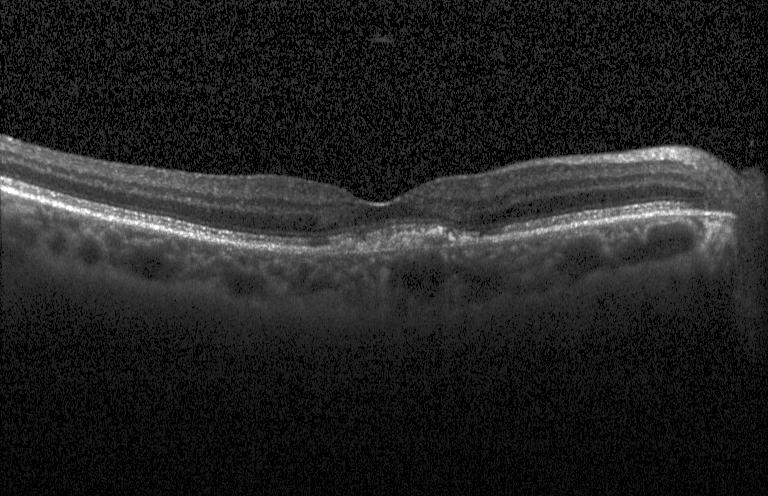

Optical coherence tomography scan, spectral-domain optical coherence tomography, through the macula. Diagnosis: a choroidal neovascular membrane.